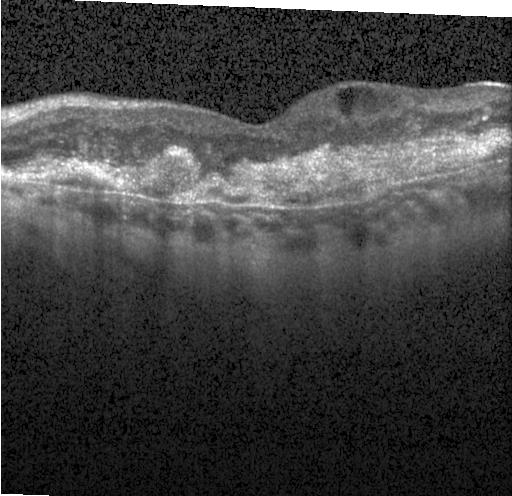
OCT B-scan. Diagnosis: choroidal neovascularization (CNV).